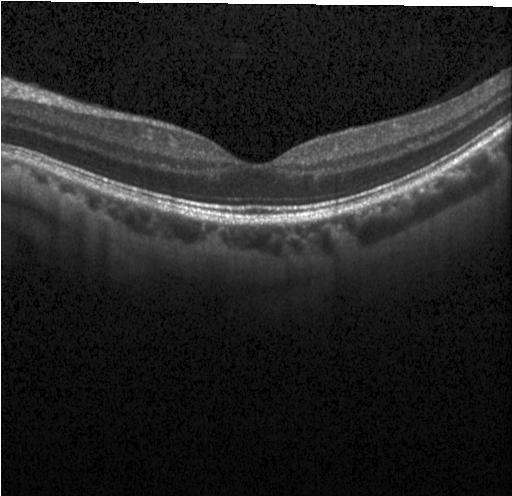 OCT B-scan showing no evidence of CNV, DME, or drusen.